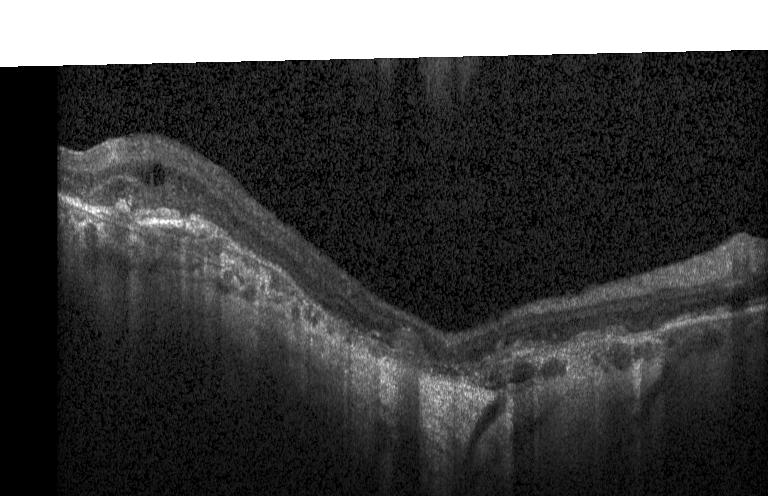 Retinal OCT B-scan.
CNV.